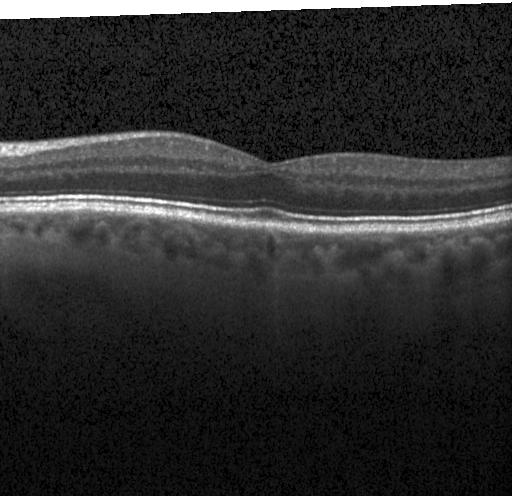 Centered on the fovea, OCT line scan. Macular OCT: no choroidal neovascularization, no diabetic macular edema, and no drusen.